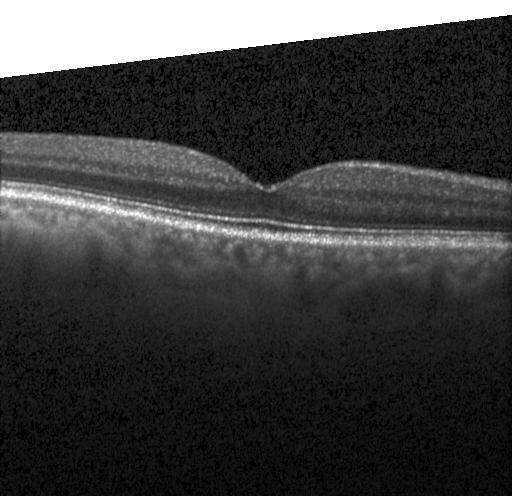
Finding: no evidence of choroidal neovascularization, diabetic macular edema, or drusen.